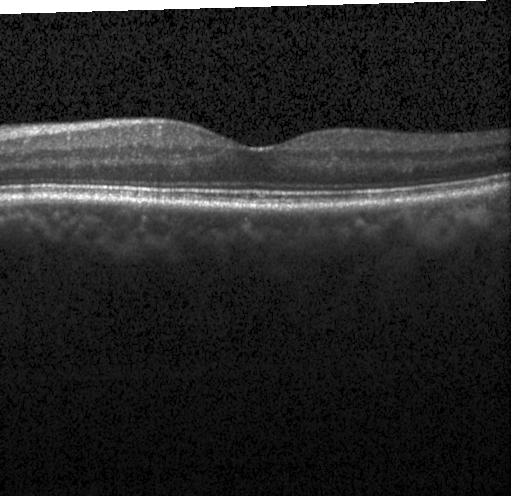

Retinal OCT cross-section
This B-scan demonstrates no choroidal neovascularization, diabetic macular edema, or drusen.